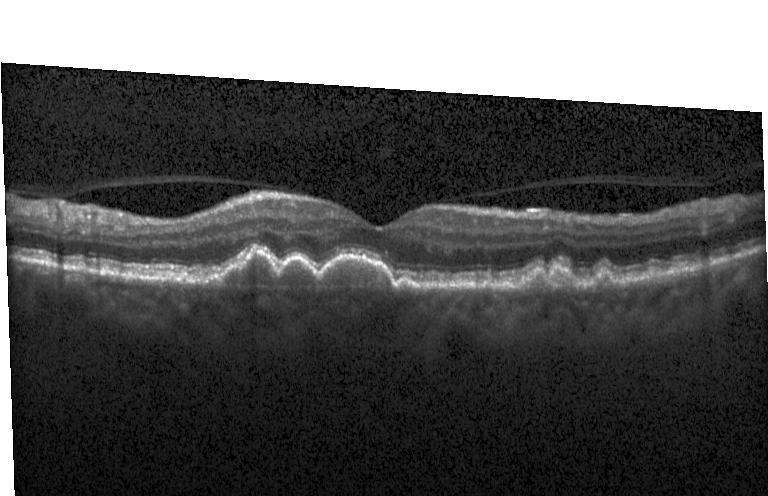 Retinal OCT cross-section showing drusen.